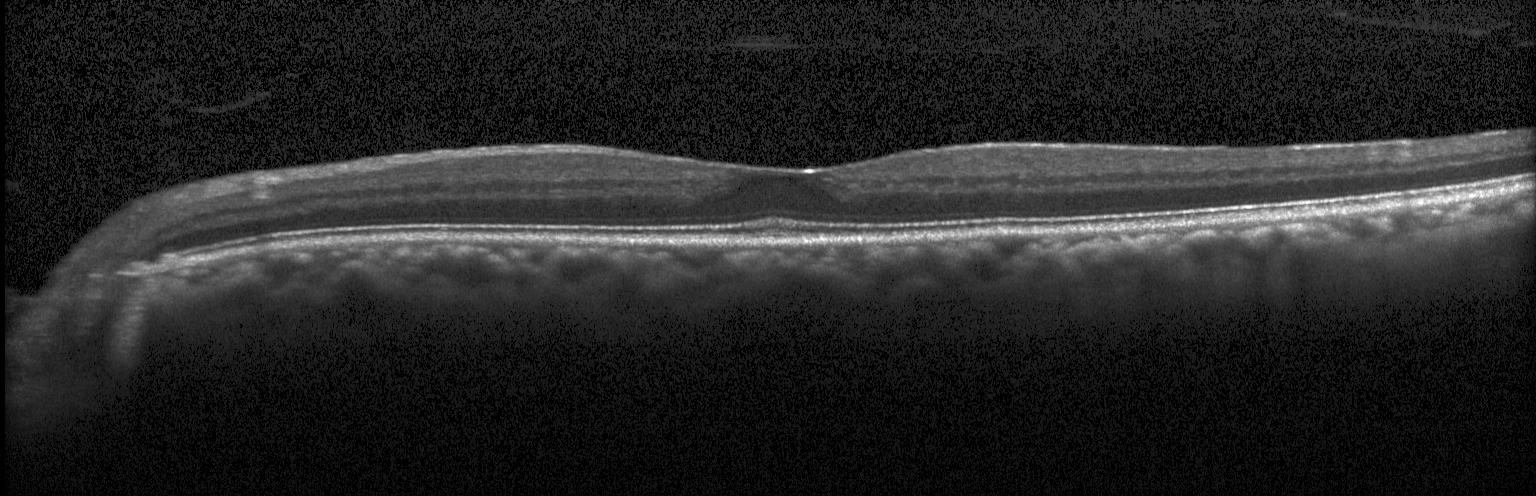
Optical coherence tomography B-scan, instrument: Heidelberg Spectralis, spectral-domain OCT, fovea-centered — Macular OCT: no CNV, no DME, and no drusen.